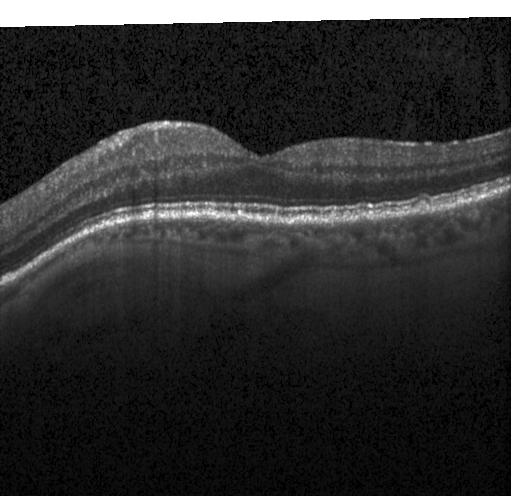 Spectral-domain OCT, optical coherence tomography scan — Assessment: drusen.